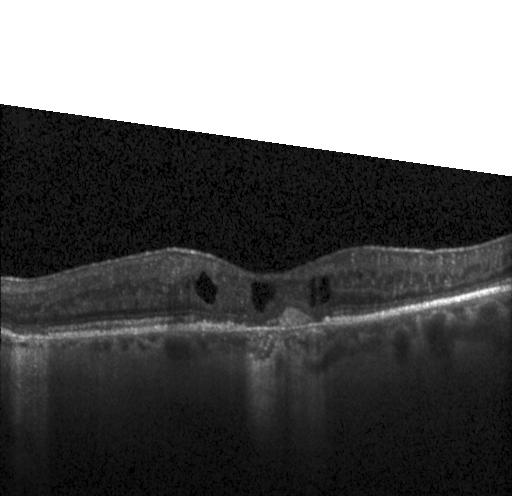
OCT line scan. The scan shows CNV.